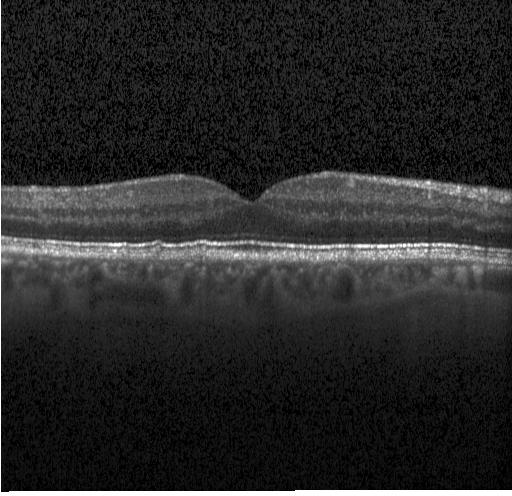

Drusen.